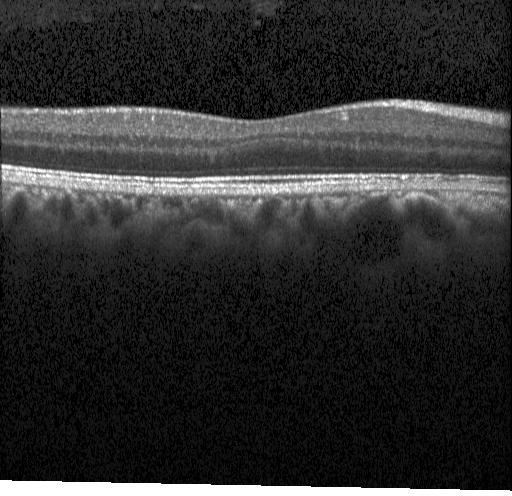 Macular OCT demonstrating neither choroidal neovascularization, diabetic macular edema, nor drusen.